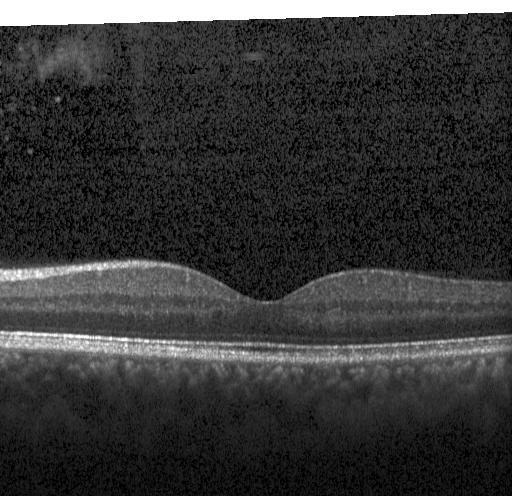 OCT B-scan. Spectral-domain optical coherence tomography.
Neither CNV, DME, nor drusen.